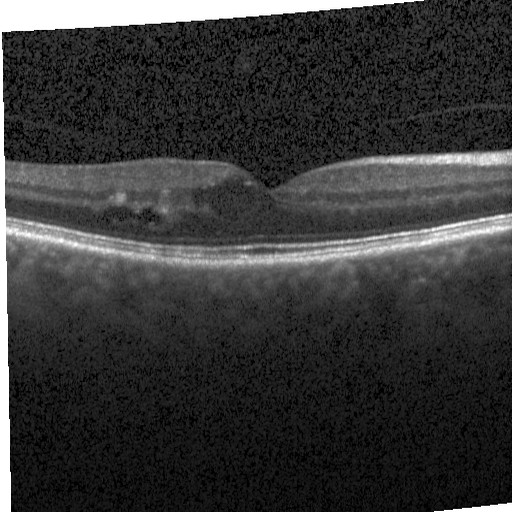

This B-scan demonstrates diabetic macular edema.